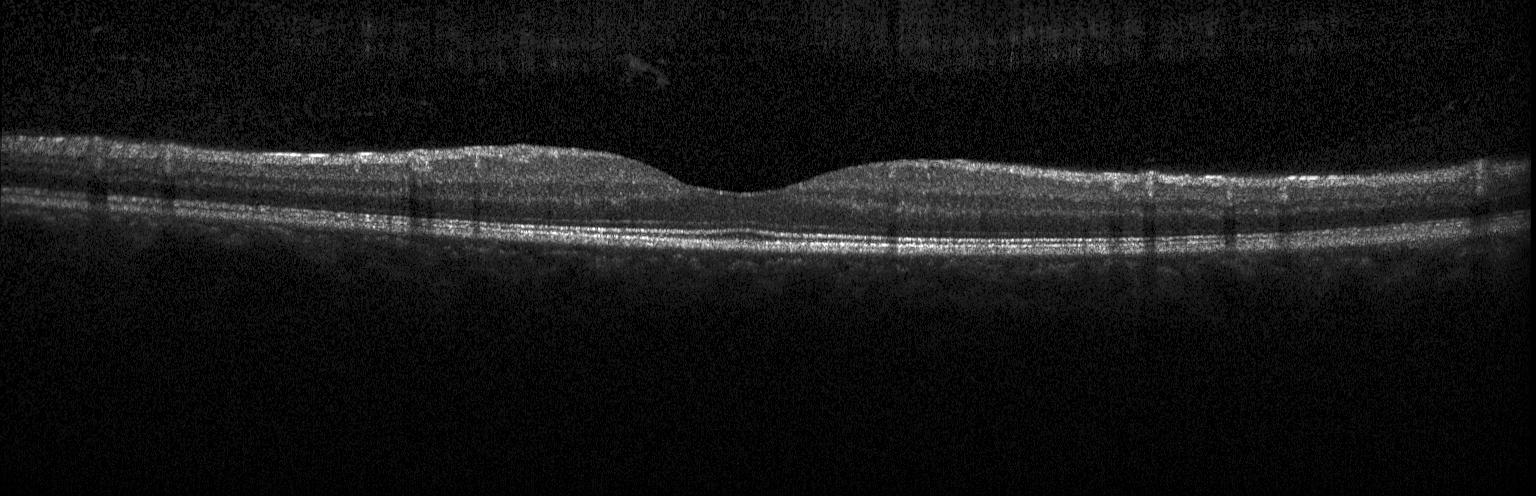 The scan shows no evidence of CNV, DME, or drusen.